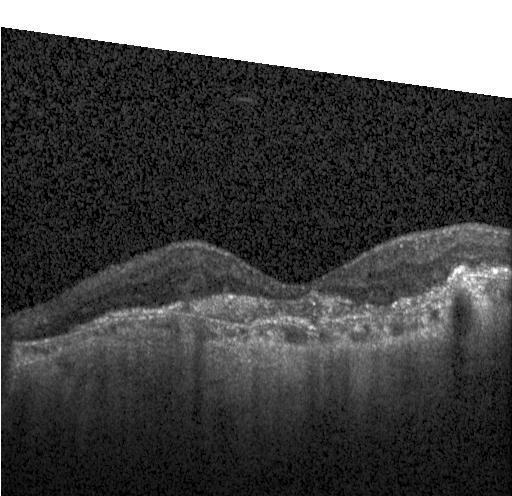 OCT B-scan. Instrument: Heidelberg Spectralis
Diagnosis: a choroidal neovascular membrane.